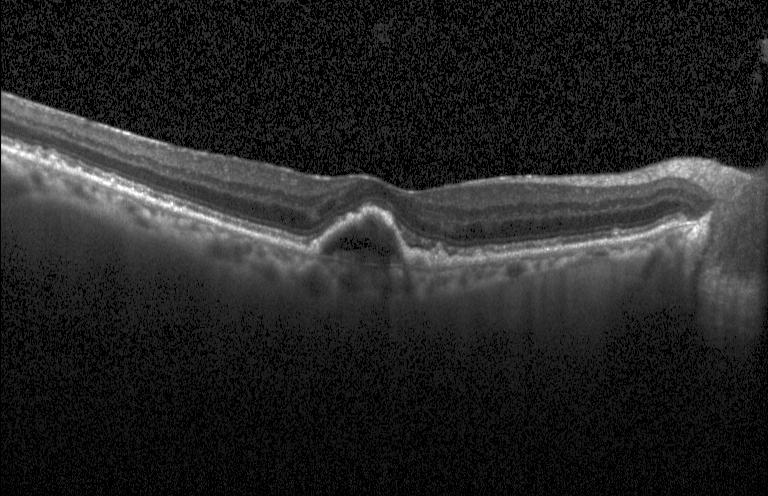

Retinal OCT B-scan, SD-OCT
Diagnosis: a choroidal neovascular membrane.